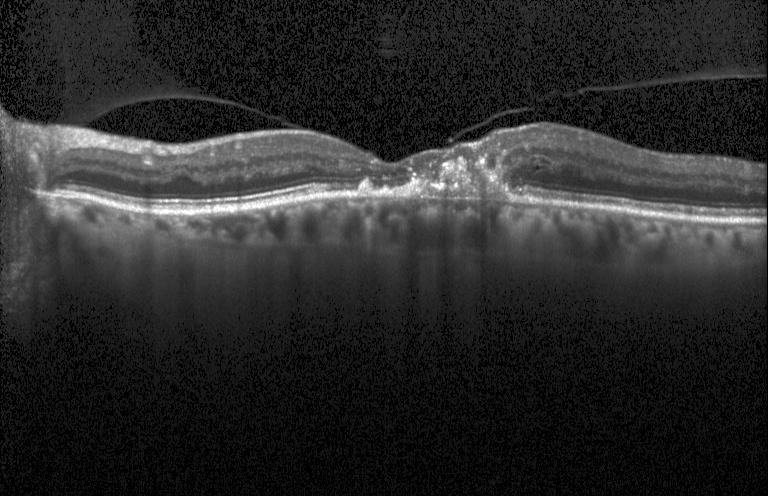

Spectral-domain OCT · OCT B-scan · Heidelberg Spectralis OCT system — The scan shows a choroidal neovascular membrane.